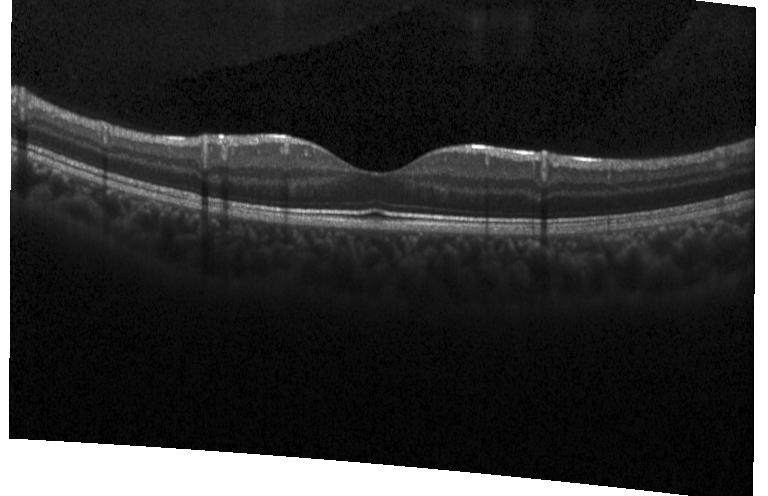

Assessment: neither choroidal neovascularization, diabetic macular edema, nor drusen.